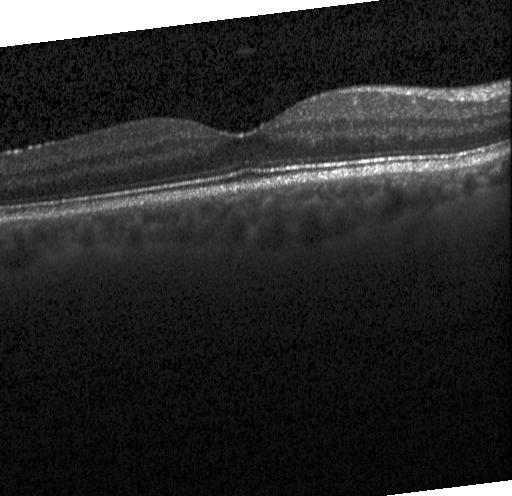 OCT scan showing no CNV, no DME, and no drusen.